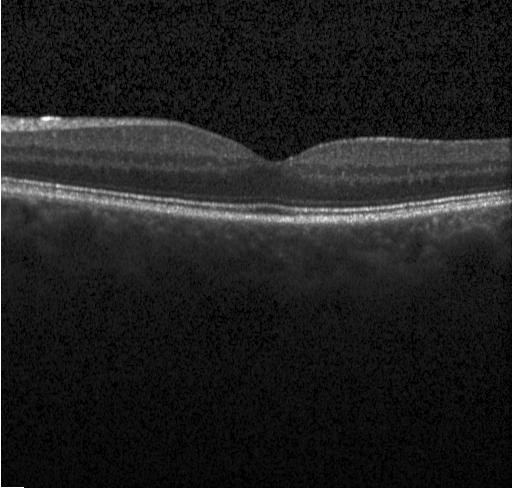
Instrument: Heidelberg Spectralis · OCT B-scan. Impression: no CNV, DME, or drusen.